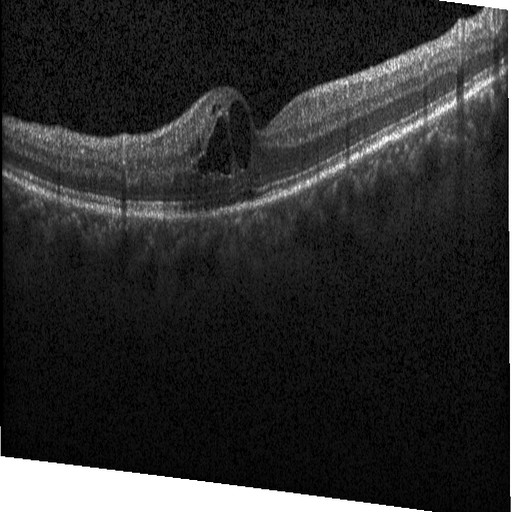 Horizontal scan through the fovea, spectral-domain OCT, retinal OCT B-scan, instrument: Heidelberg Spectralis — Impression: diabetic macular edema.